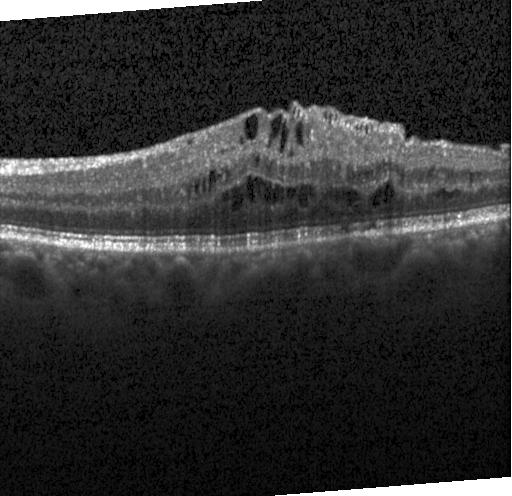

Retinal OCT cross-section, fovea-centered, spectral-domain OCT — Macular OCT: DME.